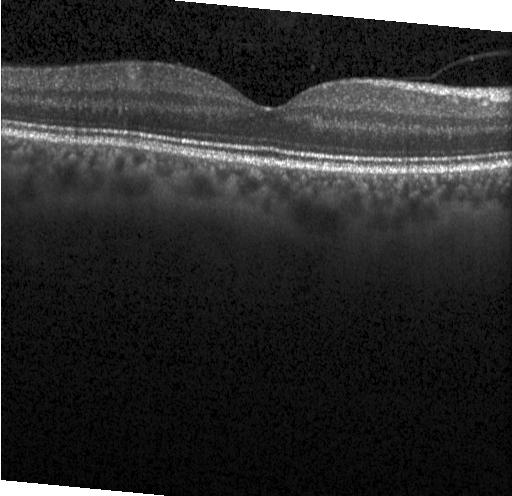 Diagnosis: no CNV, no DME, and no drusen.